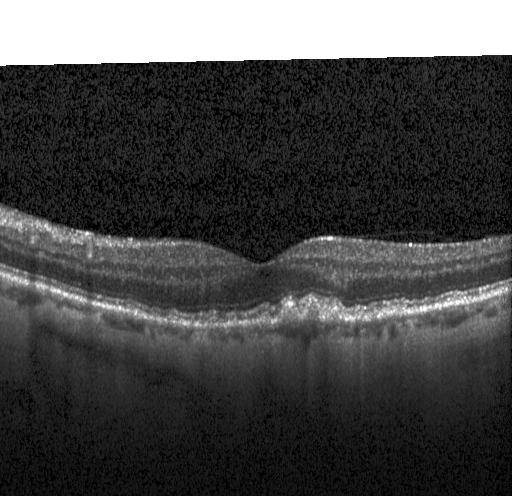
OCT B-scan showing sub-RPE drusenoid deposits.